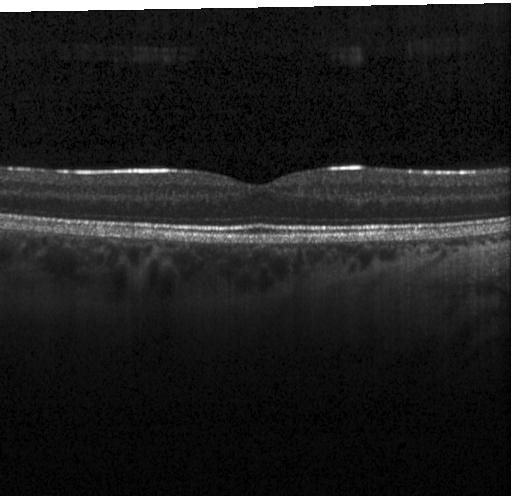
SD-OCT · Heidelberg Spectralis OCT system · optical coherence tomography B-scan — Neither choroidal neovascularization, diabetic macular edema, nor drusen.